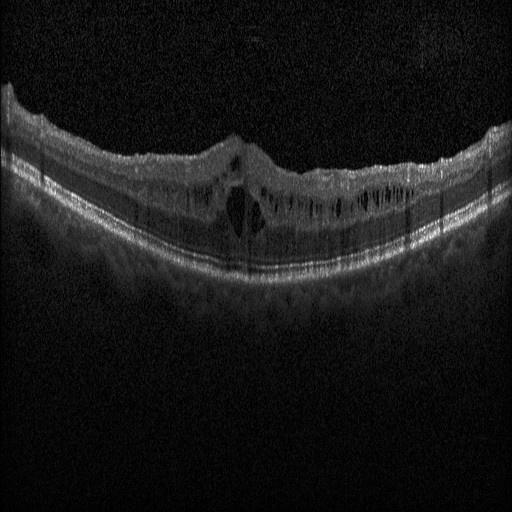
Dx: diabetic macular edema.